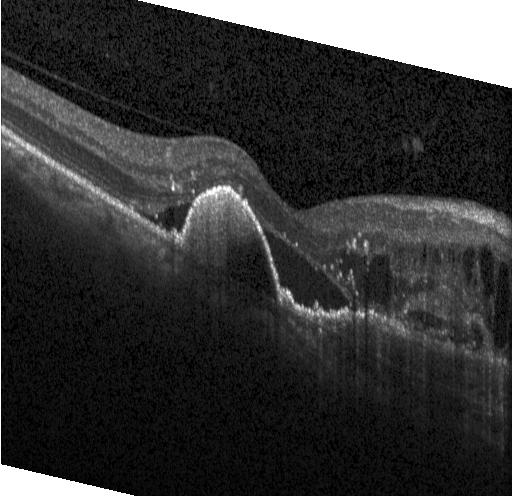
Diagnosis: choroidal neovascularization.